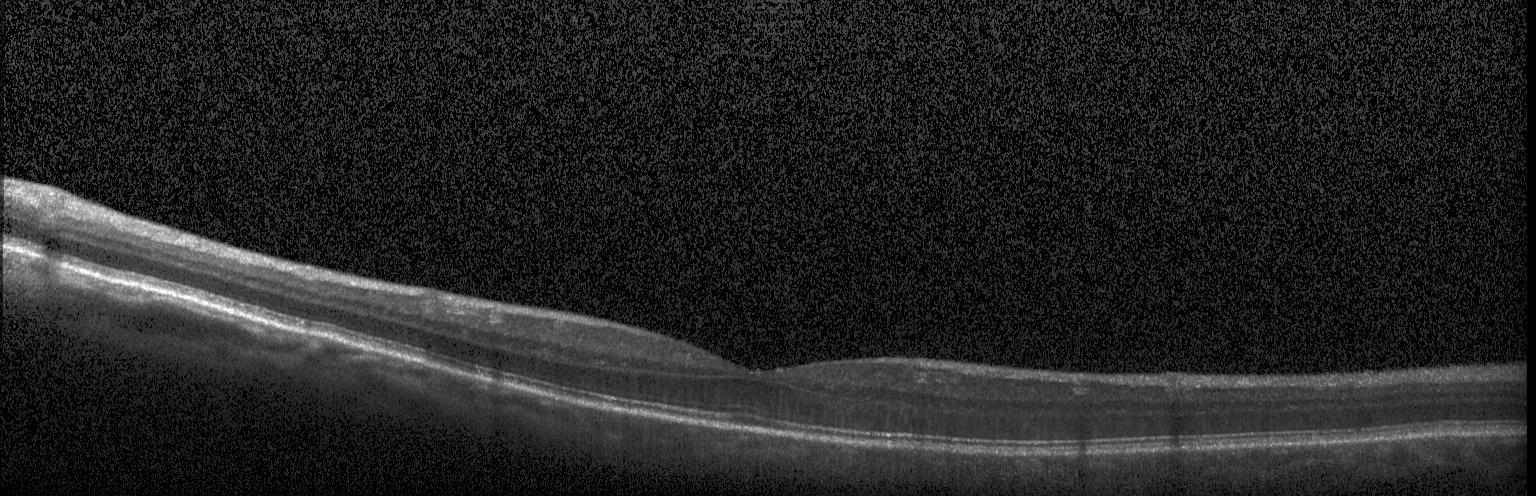
Optical coherence tomography scan — Finding: no CNV, no DME, and no drusen.